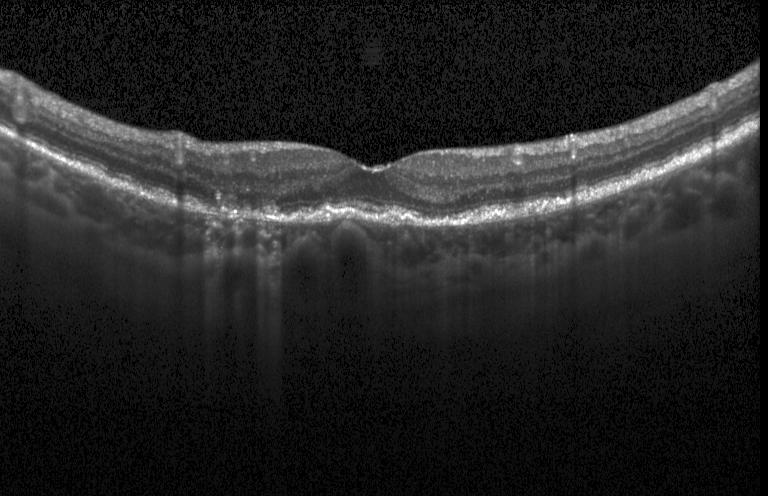
Retinal OCT cross-section. Fovea-centered — The scan shows CNV.